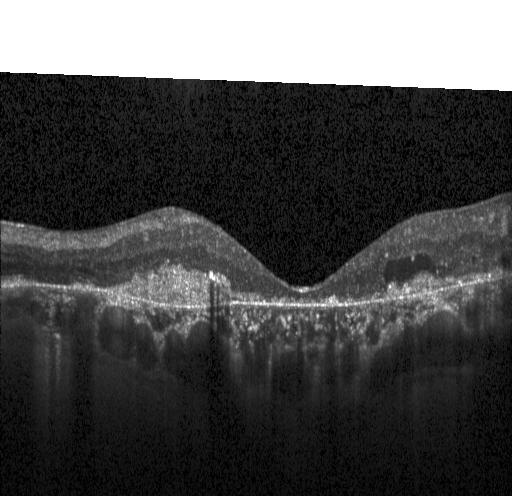

Impression: CNV.